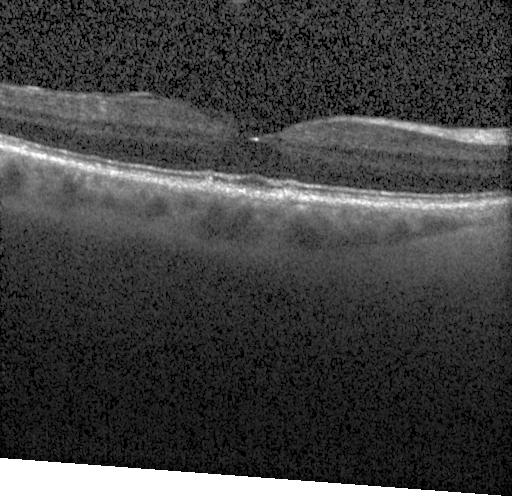

OCT line scan. This B-scan demonstrates multiple drusen.